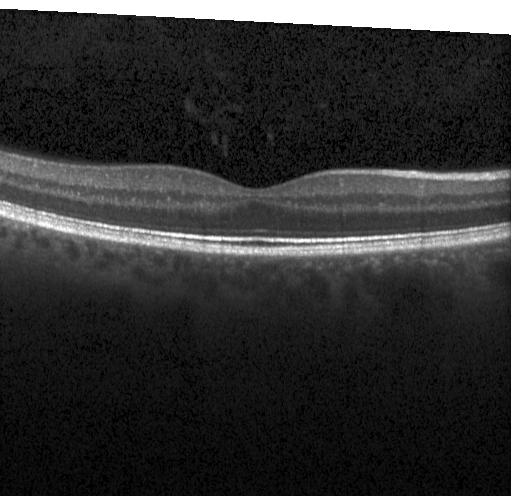 Retinal OCT cross-section · macular scan · acquired on a Heidelberg Spectralis · spectral-domain OCT
Finding: neither choroidal neovascularization, diabetic macular edema, nor drusen.